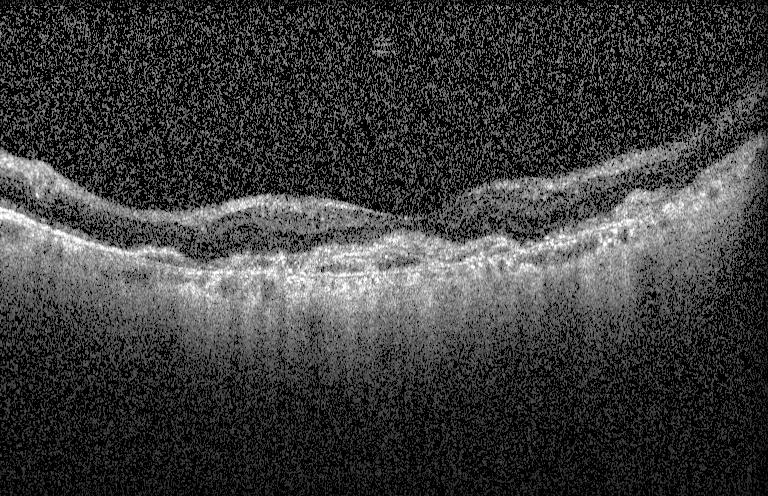 OCT line scan — A choroidal neovascular membrane.